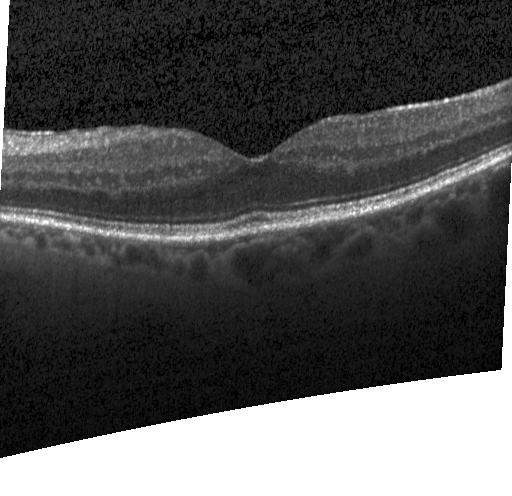
Diagnosis: no choroidal neovascularization, no diabetic macular edema, and no drusen.